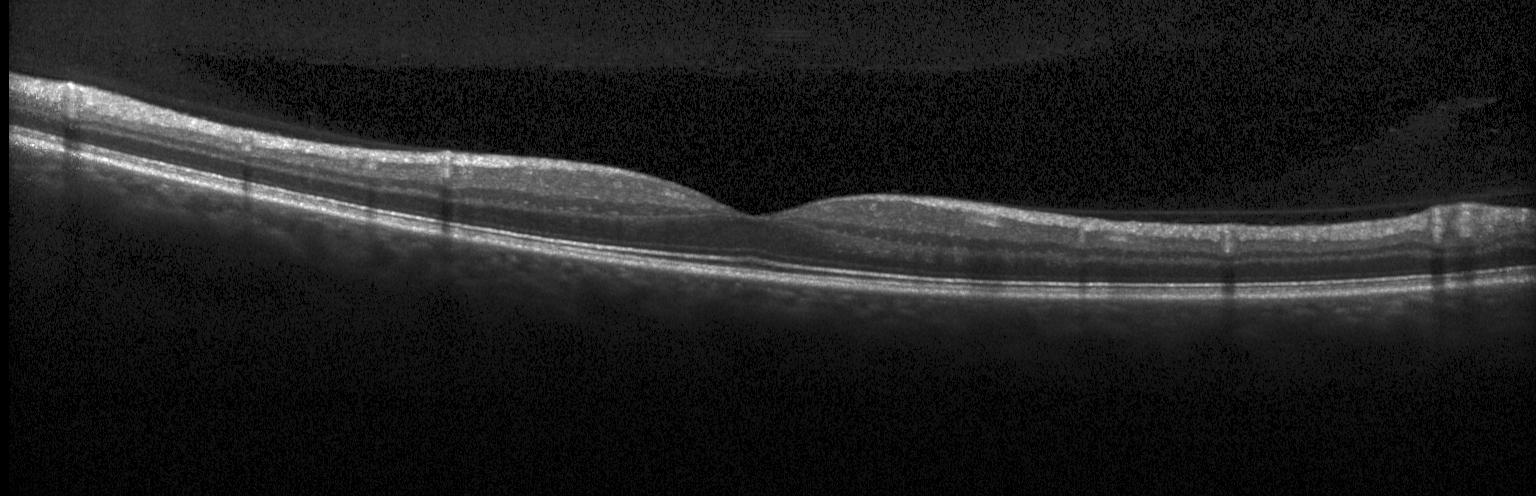
Finding: no choroidal neovascularization, no diabetic macular edema, and no drusen.